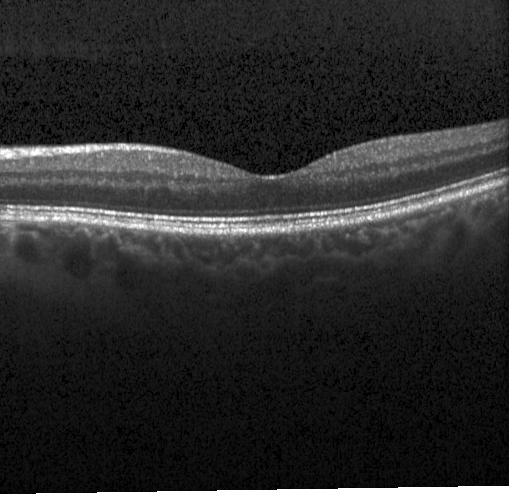

SD-OCT. Horizontal scan through the fovea. Heidelberg Spectralis. Retinal OCT B-scan. Neither CNV, DME, nor drusen.